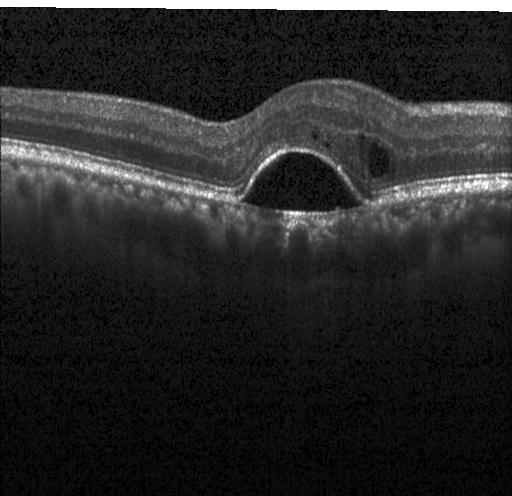 The scan shows choroidal neovascularization (CNV).